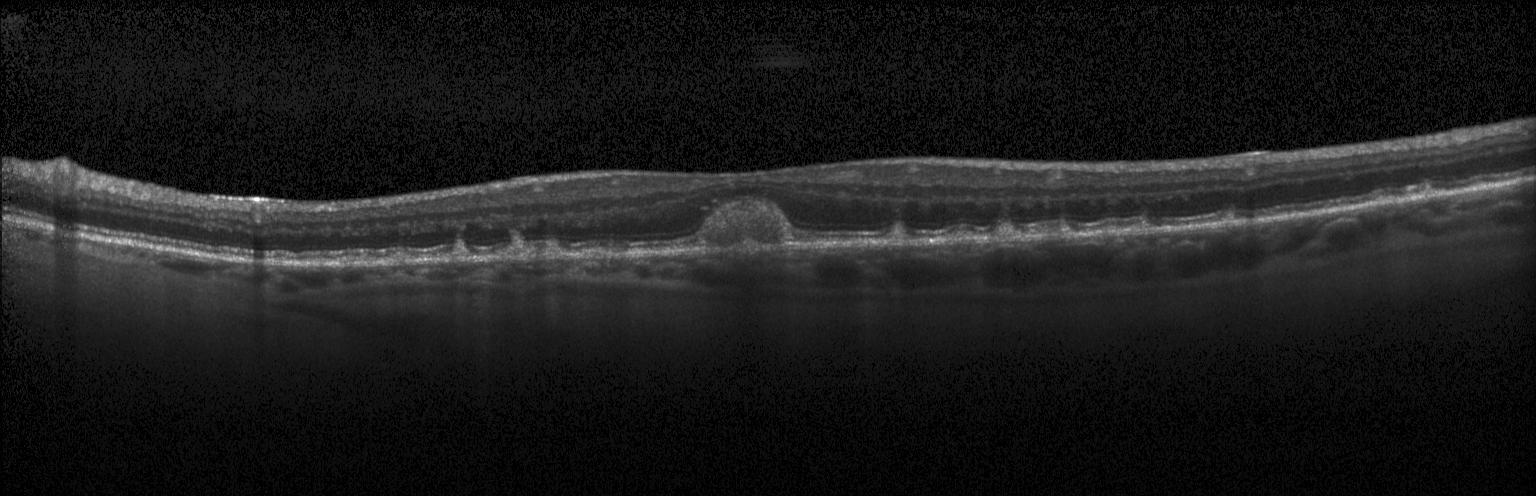

Retinal OCT cross-section showing CNV.